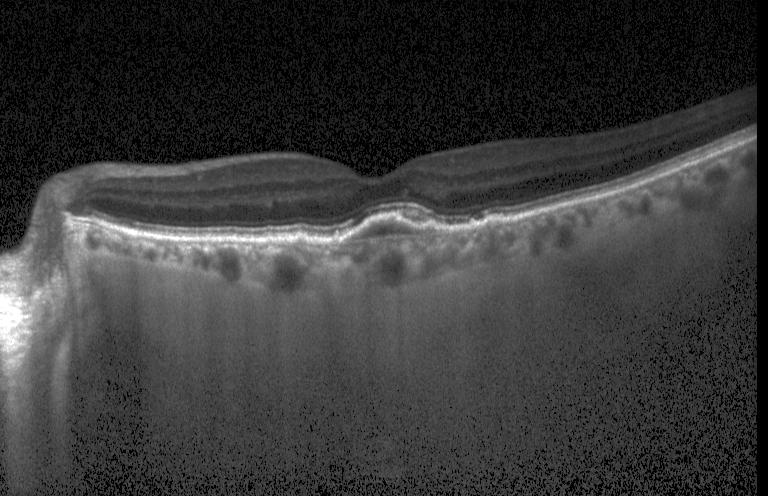

OCT finding: choroidal neovascularization.